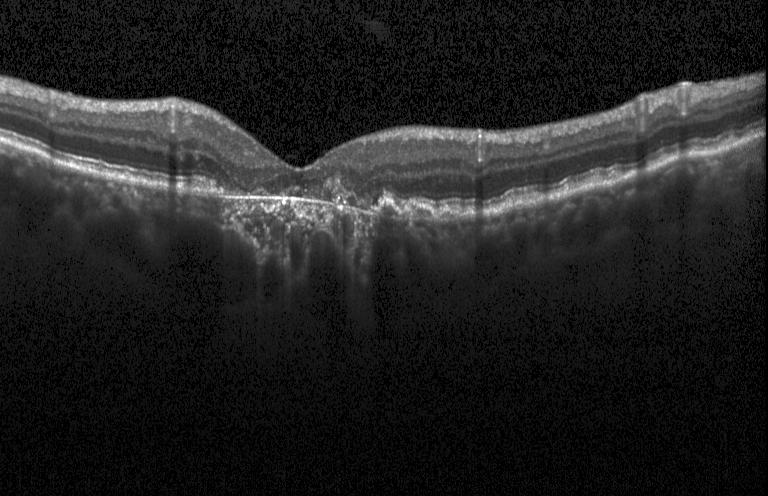
Diagnosis: a choroidal neovascular membrane.